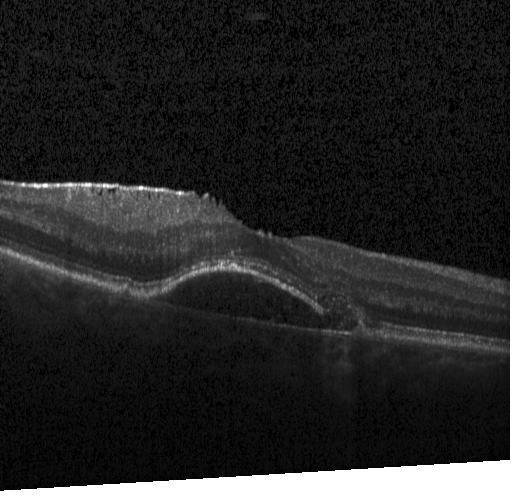
Retinal OCT cross-section, macular scan, spectral-domain optical coherence tomography. OCT finding: choroidal neovascularization.